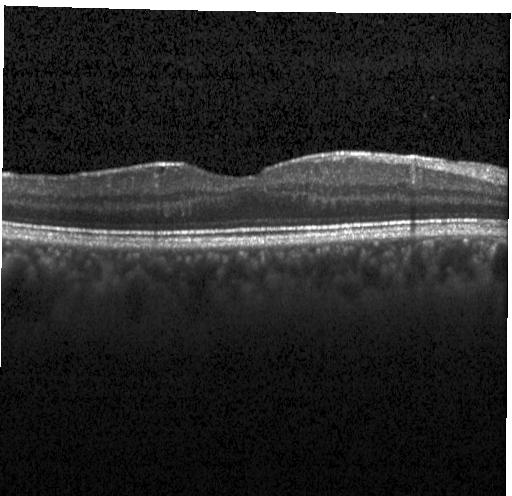 OCT B-scan; spectral-domain optical coherence tomography
Finding: no evidence of choroidal neovascularization, diabetic macular edema, or drusen.